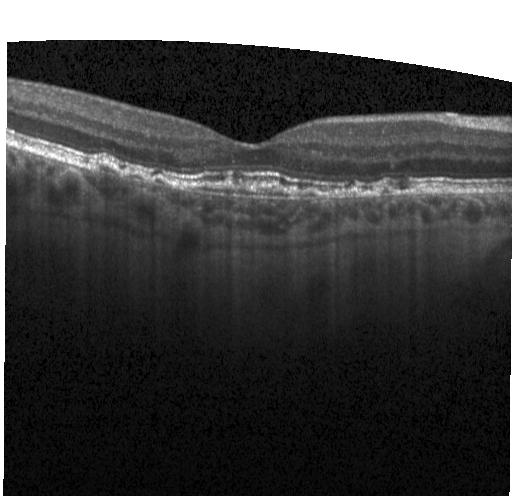
Acquired on a Heidelberg Spectralis · OCT B-scan · fovea-centered · SD-OCT.
Finding: a choroidal neovascular membrane.